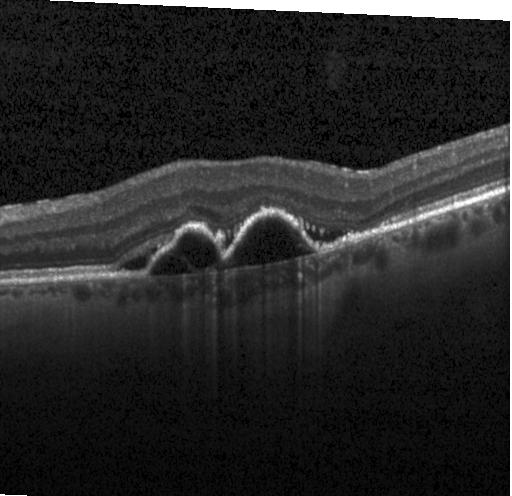
Spectral-domain OCT B-scan: a choroidal neovascular membrane.